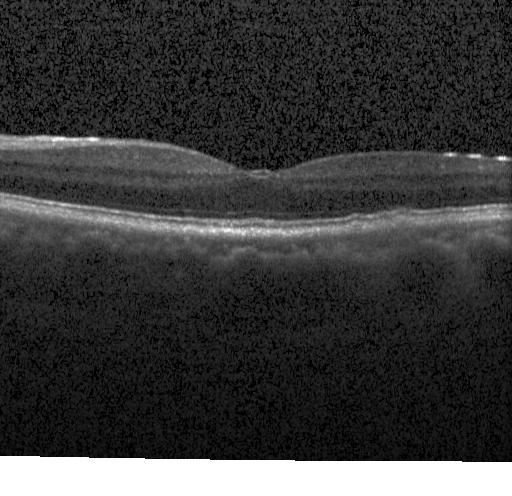
Spectral-domain optical coherence tomography; retinal OCT B-scan; instrument: Heidelberg Spectralis
Diagnosis: sub-RPE drusenoid deposits.